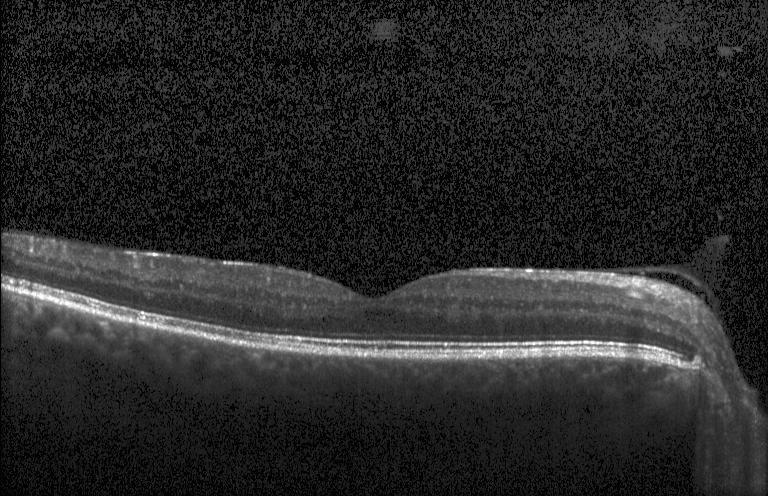
Fovea-centered · instrument: Heidelberg Spectralis · spectral-domain OCT · OCT line scan. Diagnosis: no choroidal neovascularization, diabetic macular edema, or drusen.